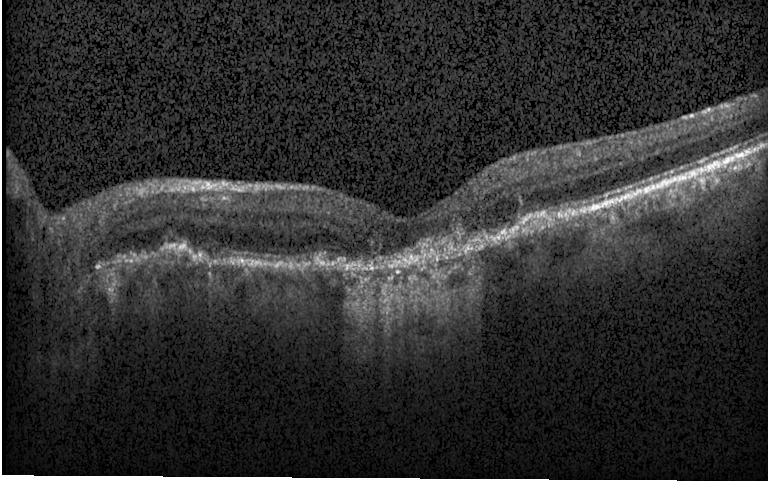
Optical coherence tomography B-scan. Macular scan — Diagnosis: CNV.